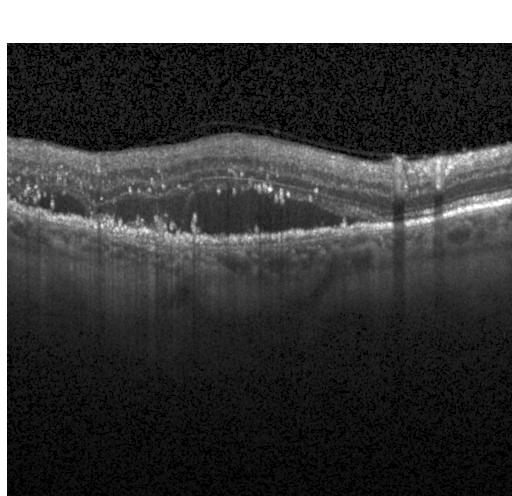 Spectral-domain optical coherence tomography · retinal OCT B-scan — Finding: a choroidal neovascular membrane.